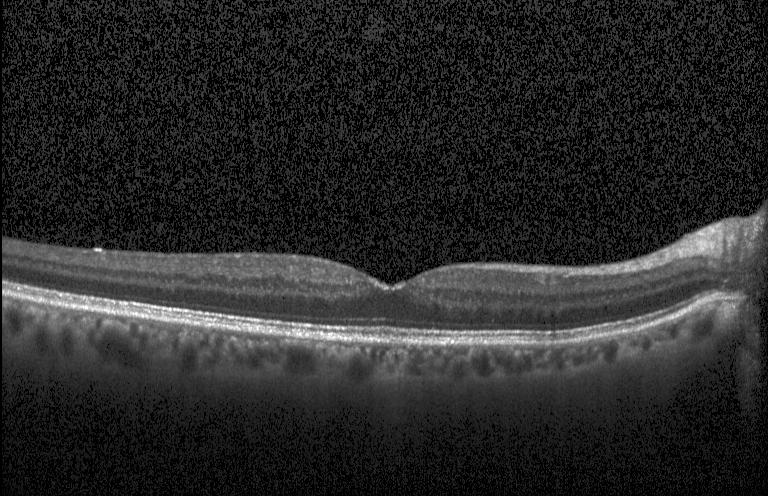
Macular OCT: no choroidal neovascularization, diabetic macular edema, or drusen.